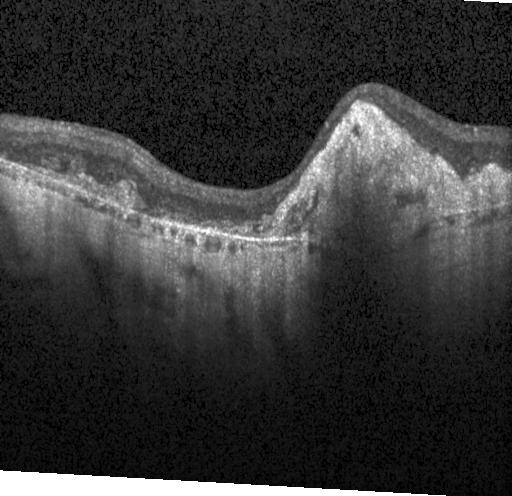 SD-OCT; acquired on a Heidelberg Spectralis; through the macula; retinal OCT cross-section. Assessment: a choroidal neovascular membrane.